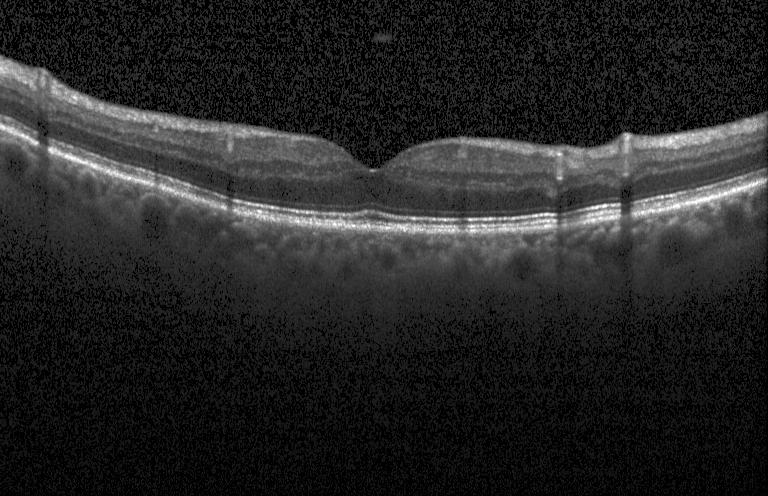

Retinal OCT cross-section. OCT finding: no choroidal neovascularization, diabetic macular edema, or drusen.